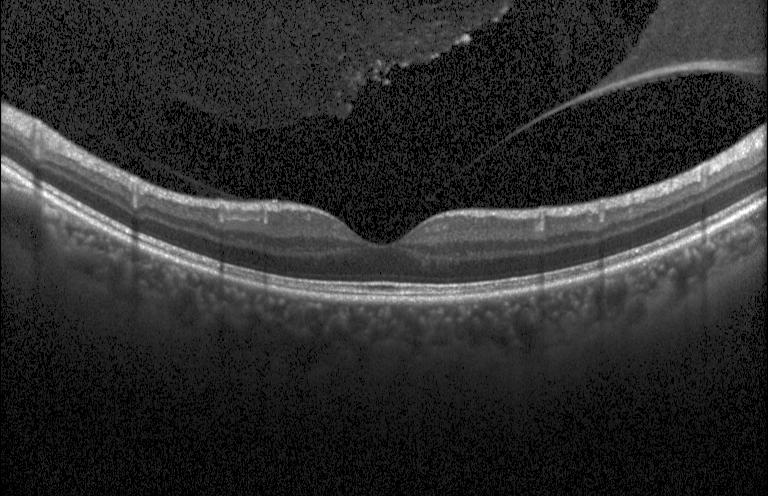
Heidelberg Spectralis · OCT line scan — Finding: no choroidal neovascularization, diabetic macular edema, or drusen.